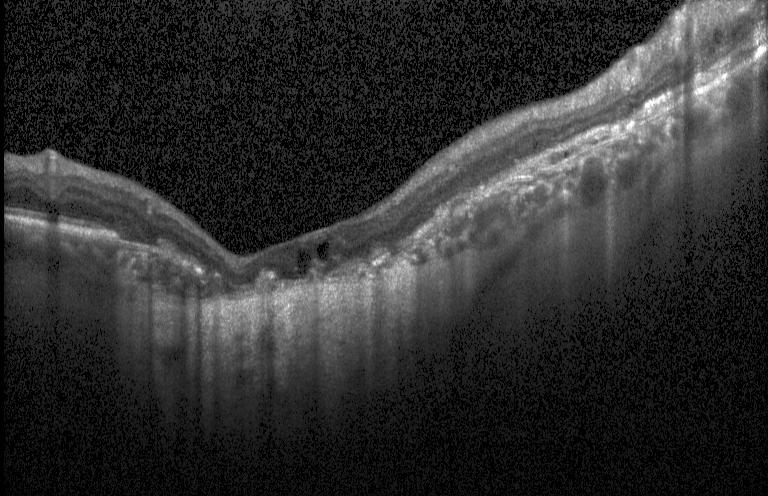
The scan shows choroidal neovascularization.